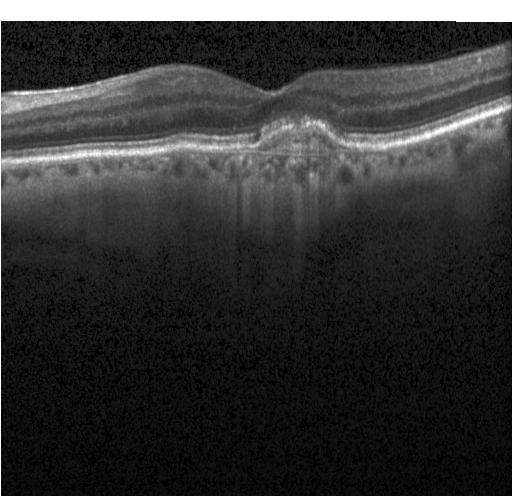 Retinal OCT cross-section showing choroidal neovascularization.